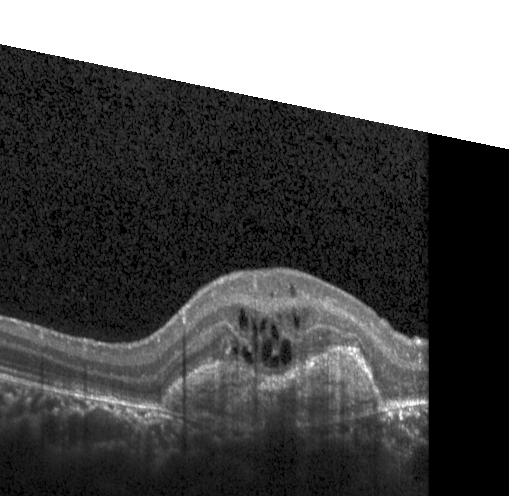
Optical coherence tomography B-scan
This B-scan demonstrates a choroidal neovascular membrane.